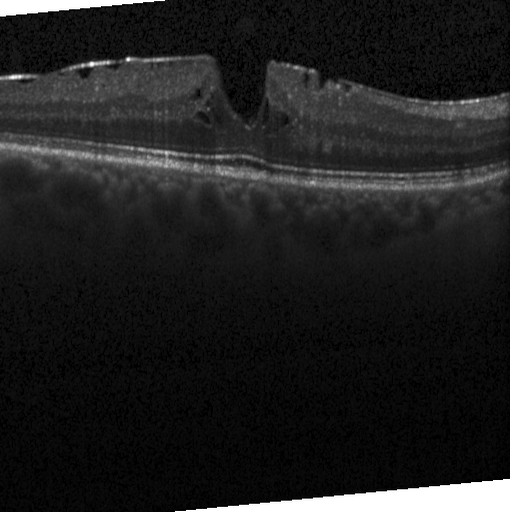 Impression: diabetic macular edema.